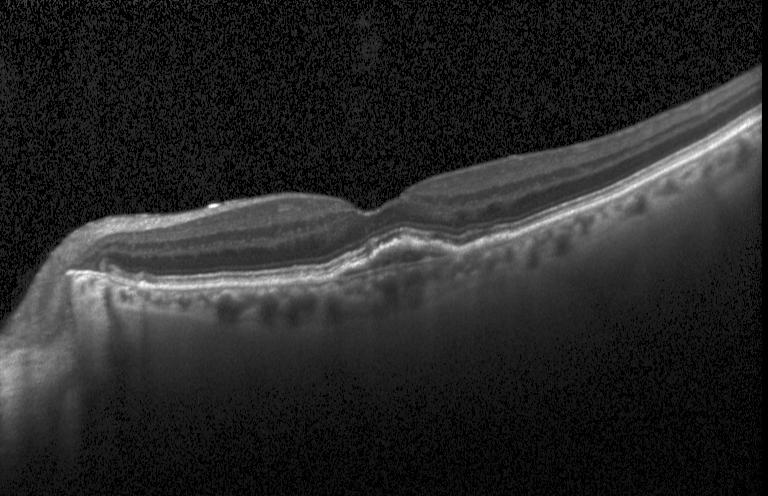 Retinal OCT cross-section showing CNV.